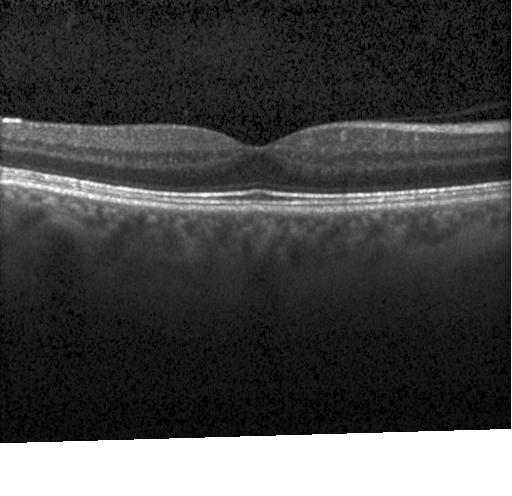
OCT B-scan; spectral-domain optical coherence tomography; Heidelberg Spectralis — Diagnosis: no evidence of choroidal neovascularization, diabetic macular edema, or drusen.